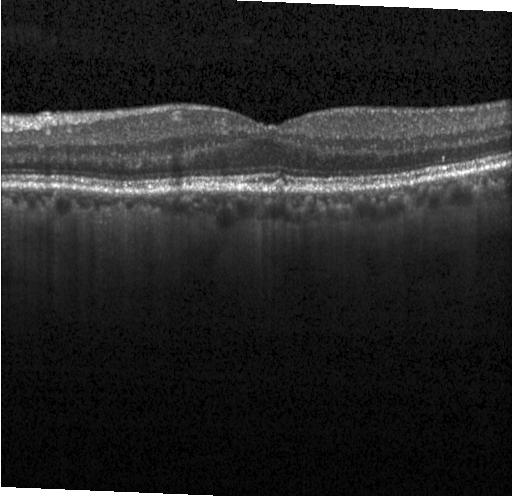 Retinal OCT cross-section, spectral-domain optical coherence tomography, instrument: Heidelberg Spectralis, horizontal scan through the fovea.
Diagnosis: multiple drusen.